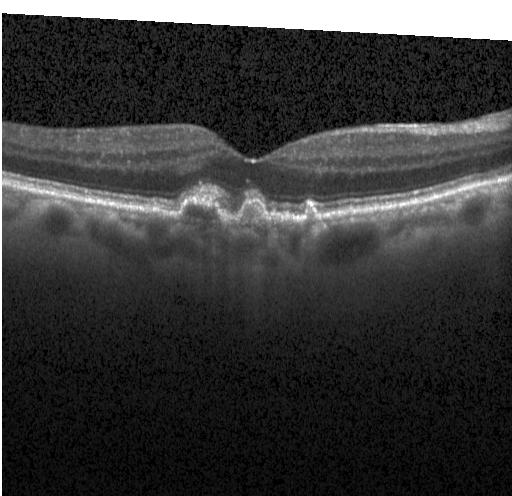
Retinal OCT B-scan · acquired on a Heidelberg Spectralis · spectral-domain optical coherence tomography · through the macula
Assessment: CNV.